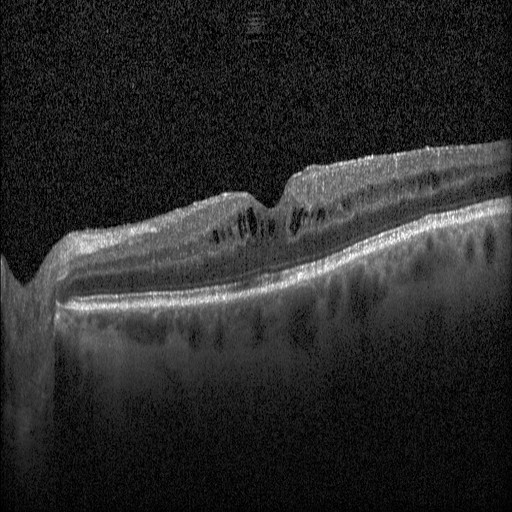 OCT finding: DME.